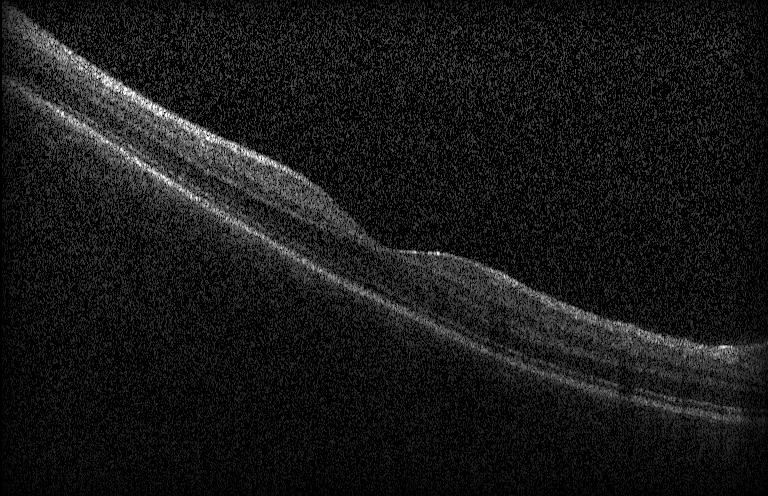

OCT finding: no CNV, no DME, and no drusen.